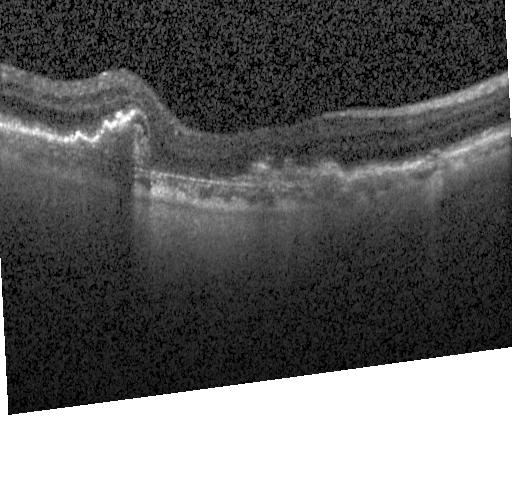

Finding: choroidal neovascularization.